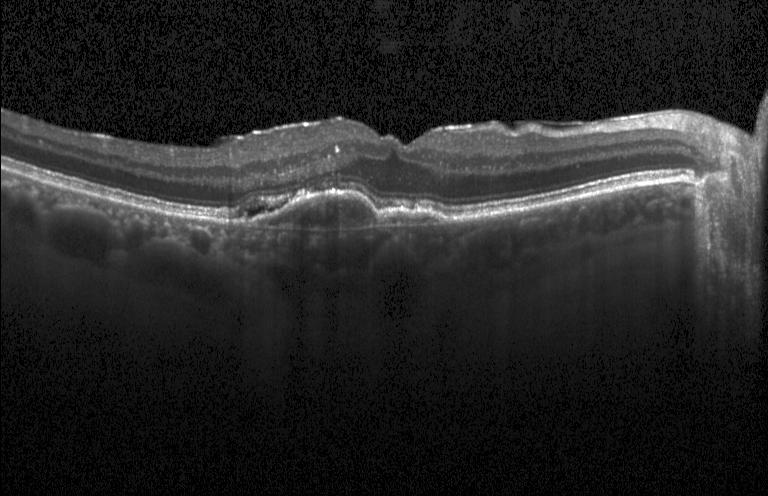
Assessment: choroidal neovascularization.